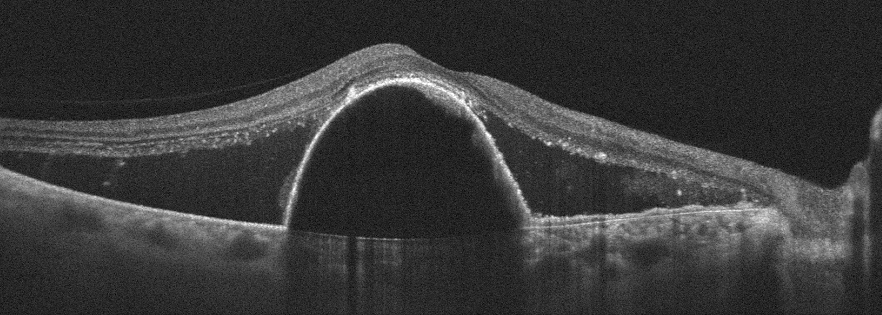 OD, retinal OCT cross-section
The scan shows age-related macular degeneration.